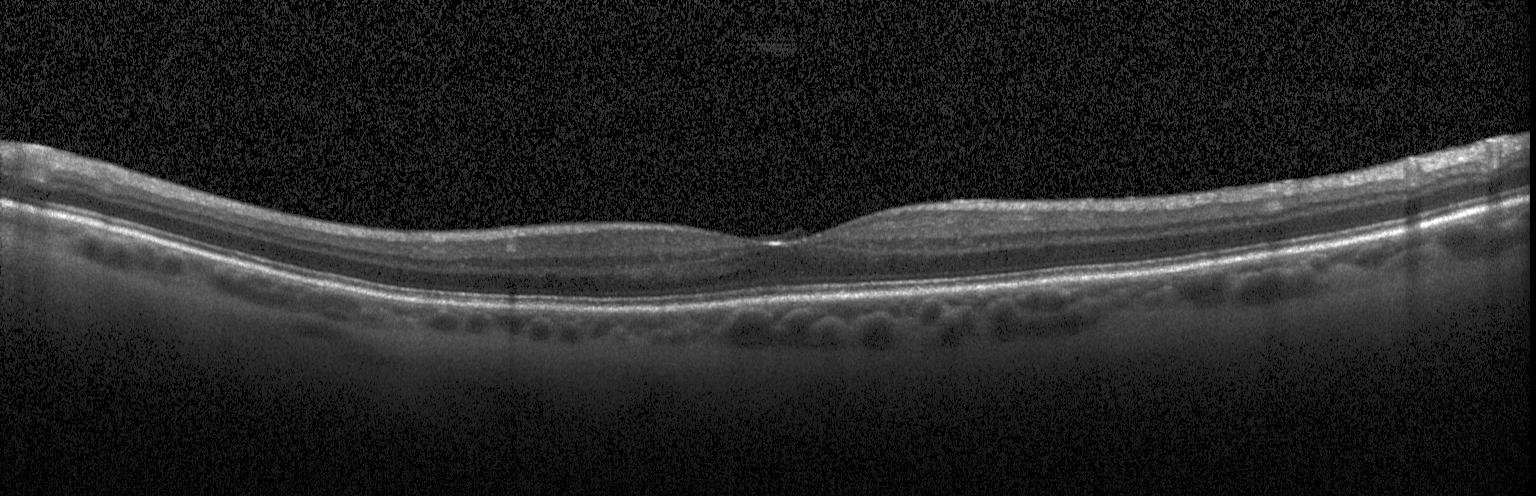 Spectral-domain OCT · optical coherence tomography scan · Heidelberg Spectralis · centered on the fovea
OCT finding: no CNV, DME, or drusen.